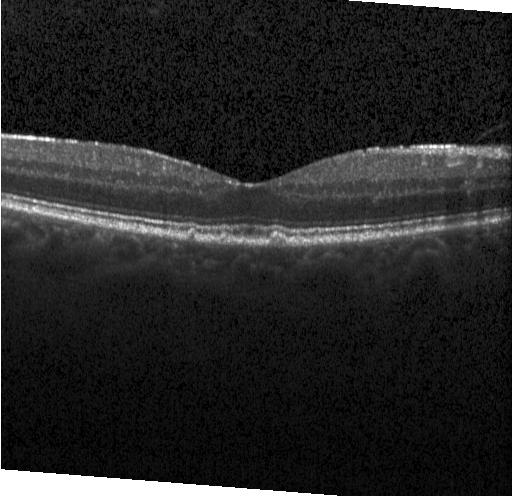
Horizontal scan through the fovea · optical coherence tomography B-scan · instrument: Heidelberg Spectralis
Diagnosis: drusen.